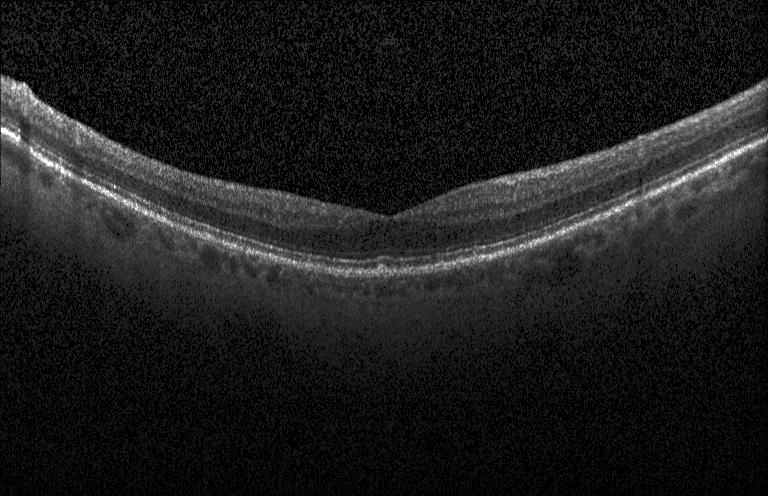

Retinal OCT B-scan.
Finding: sub-RPE drusenoid deposits.